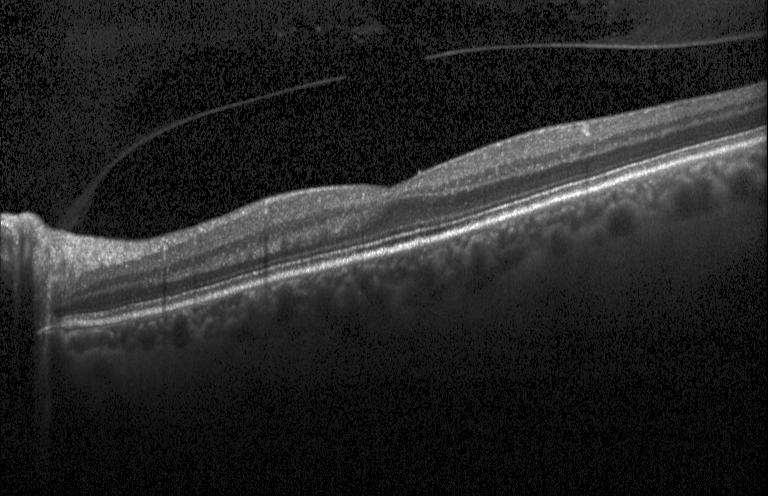

Spectral-domain OCT B-scan: no CNV, DME, or drusen.